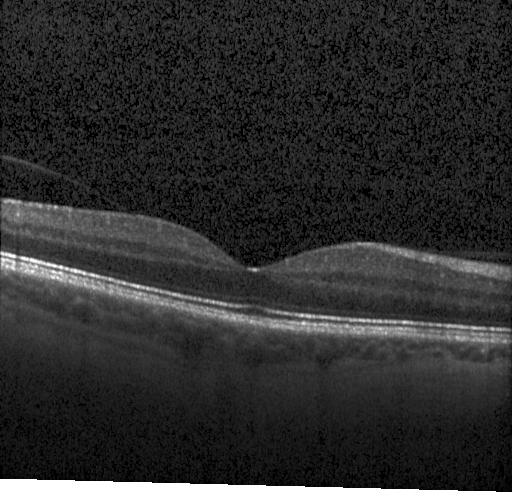
Macular OCT demonstrating no evidence of choroidal neovascularization, diabetic macular edema, or drusen.